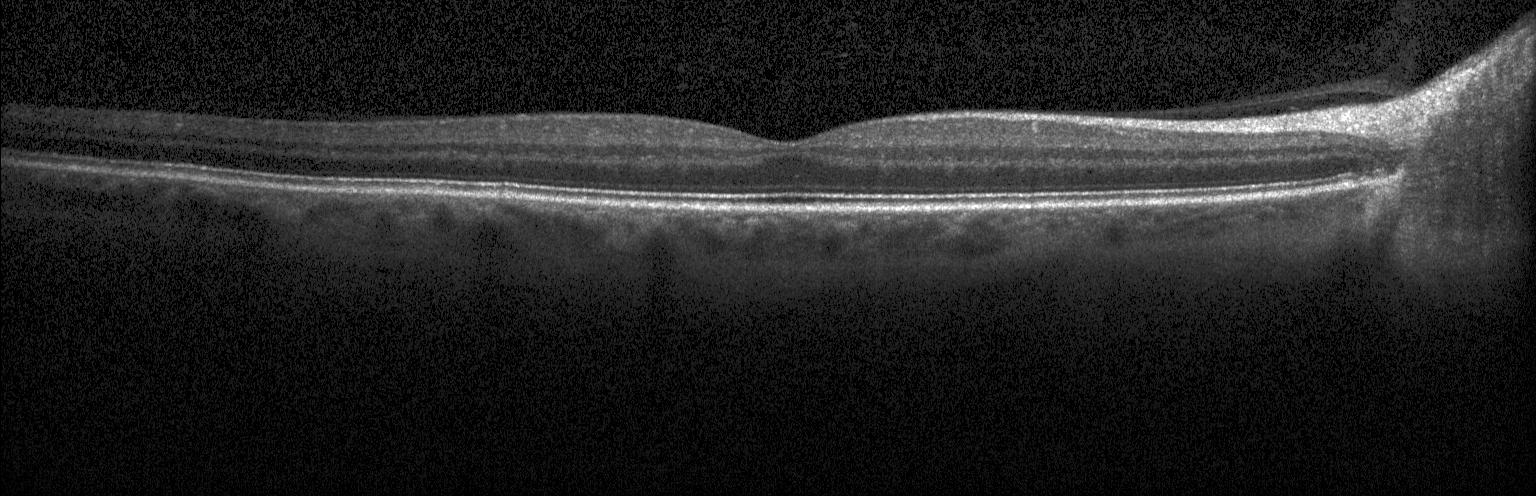

Retinal OCT B-scan — Diagnosis: neither CNV, DME, nor drusen.